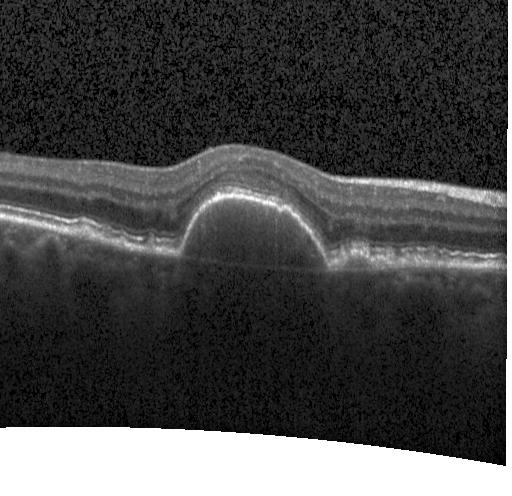

Impression: a choroidal neovascular membrane.